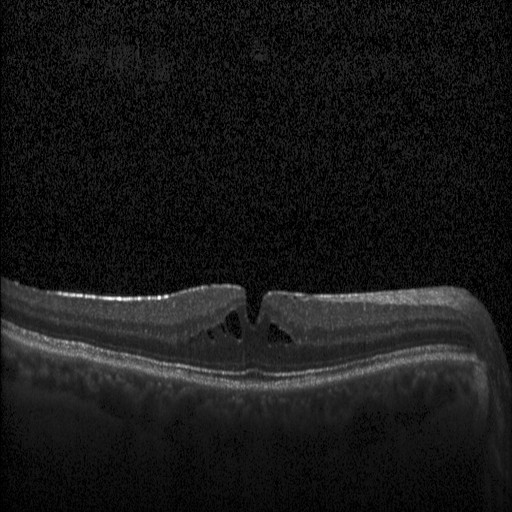 Finding: diabetic macular edema (DME).